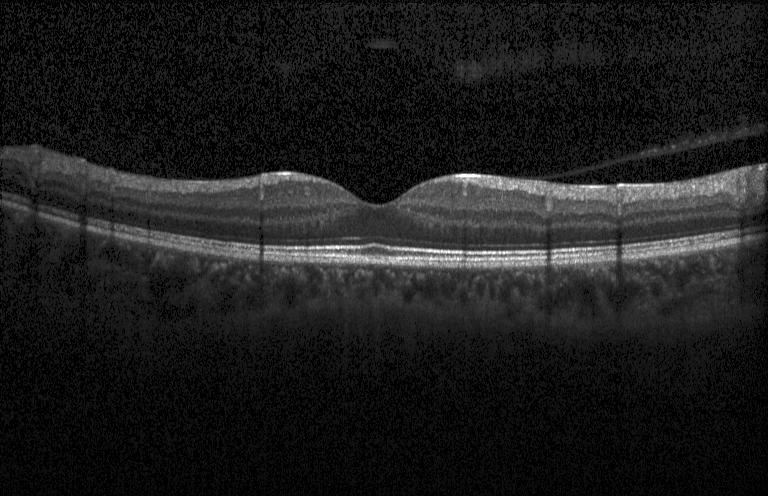 Diagnosis: no choroidal neovascularization, no diabetic macular edema, and no drusen.